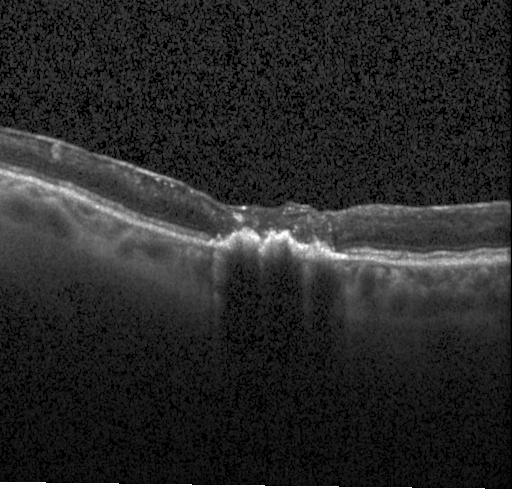

Through the macula, SD-OCT, optical coherence tomography scan, acquired on a Heidelberg Spectralis.
Diagnosis: CNV.